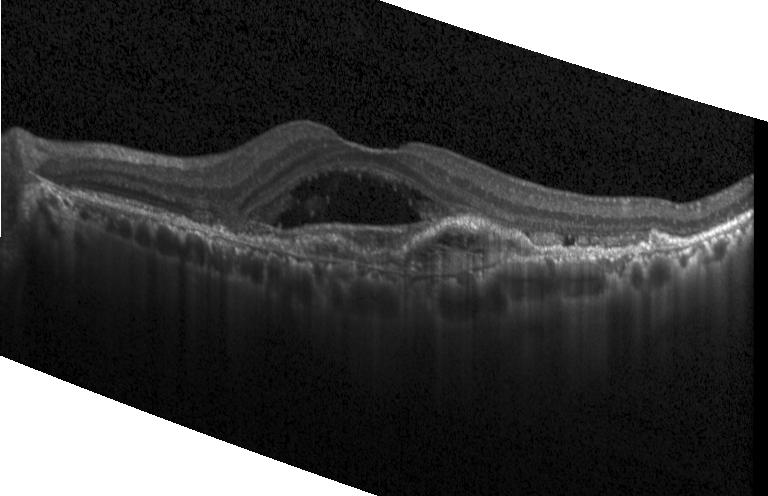 Assessment: a choroidal neovascular membrane.